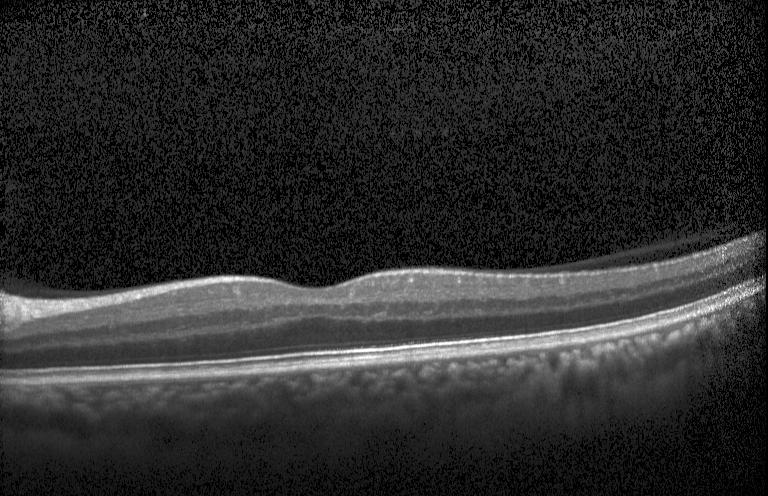 Spectral-domain OCT B-scan: no CNV, DME, or drusen.